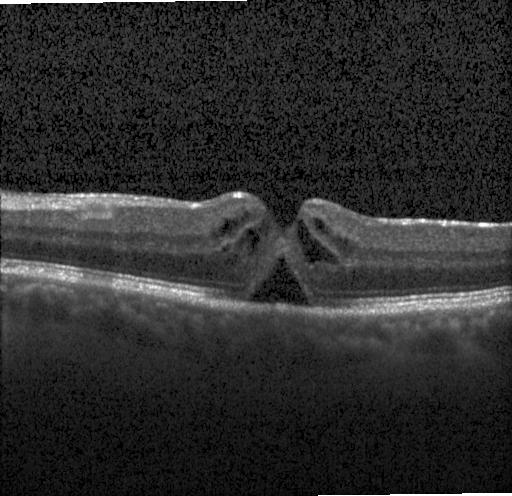 Spectral-domain OCT B-scan: diabetic macular edema.